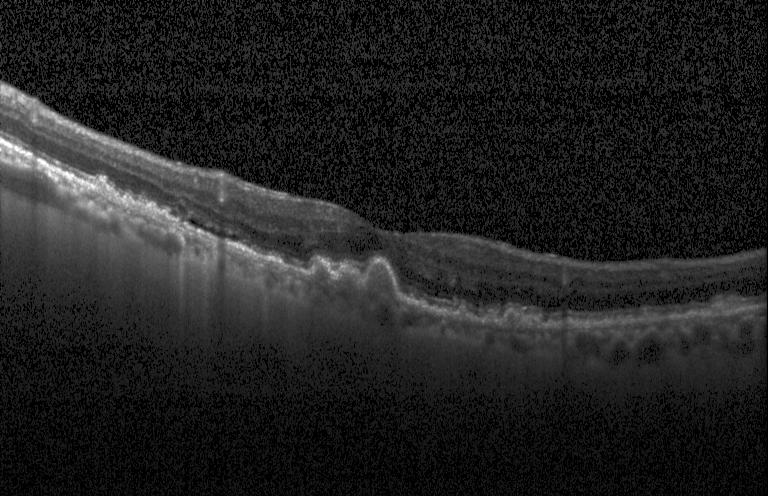

Spectral-domain OCT B-scan: choroidal neovascularization.